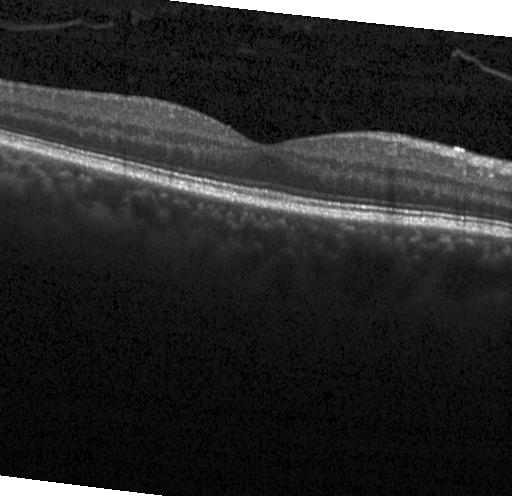 Macular scan · acquired on a Heidelberg Spectralis · OCT line scan · spectral-domain optical coherence tomography. The scan shows no choroidal neovascularization, diabetic macular edema, or drusen.